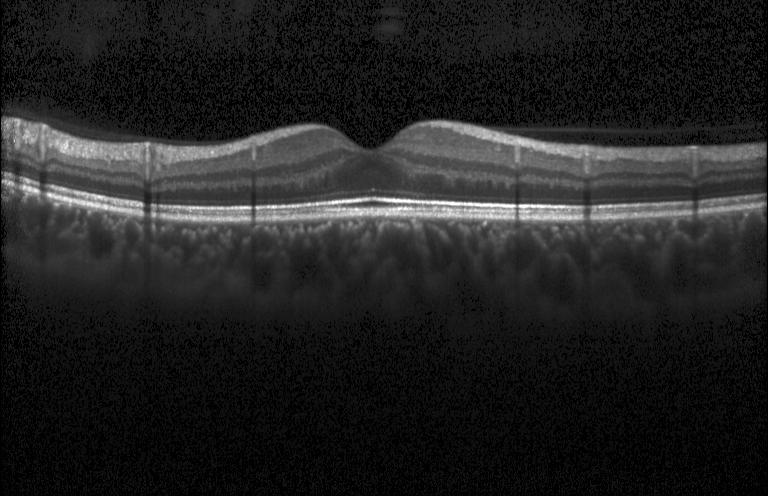 Heidelberg Spectralis · centered on the fovea · optical coherence tomography scan · spectral-domain optical coherence tomography
Diagnosis: no choroidal neovascularization, no diabetic macular edema, and no drusen.